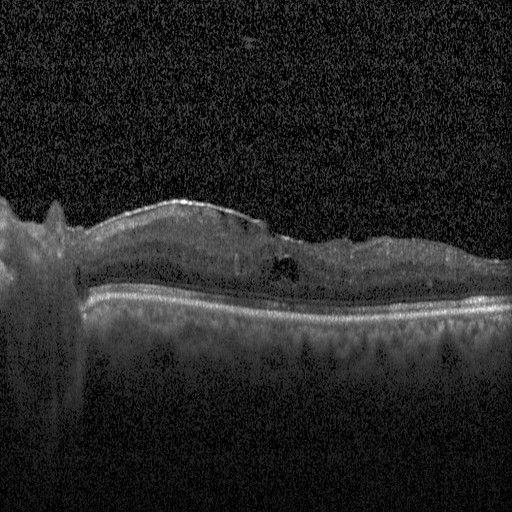

Fovea-centered · optical coherence tomography scan — Diagnosis: diabetic macular edema (DME).